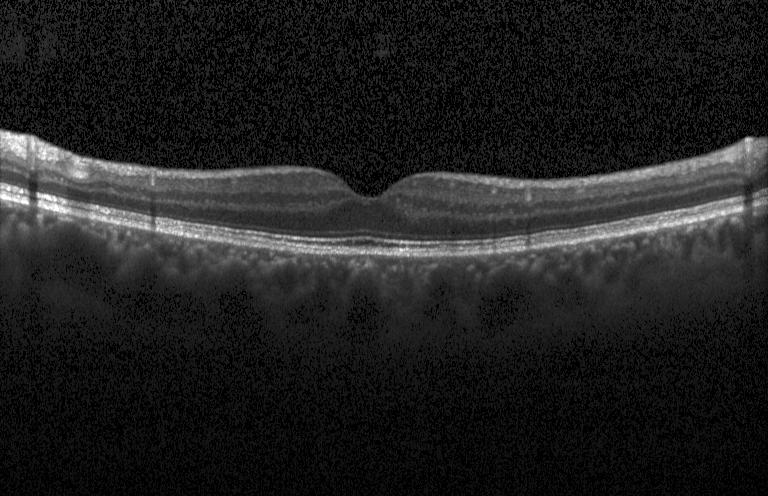 SD-OCT, OCT B-scan.
Assessment: no choroidal neovascularization, diabetic macular edema, or drusen.